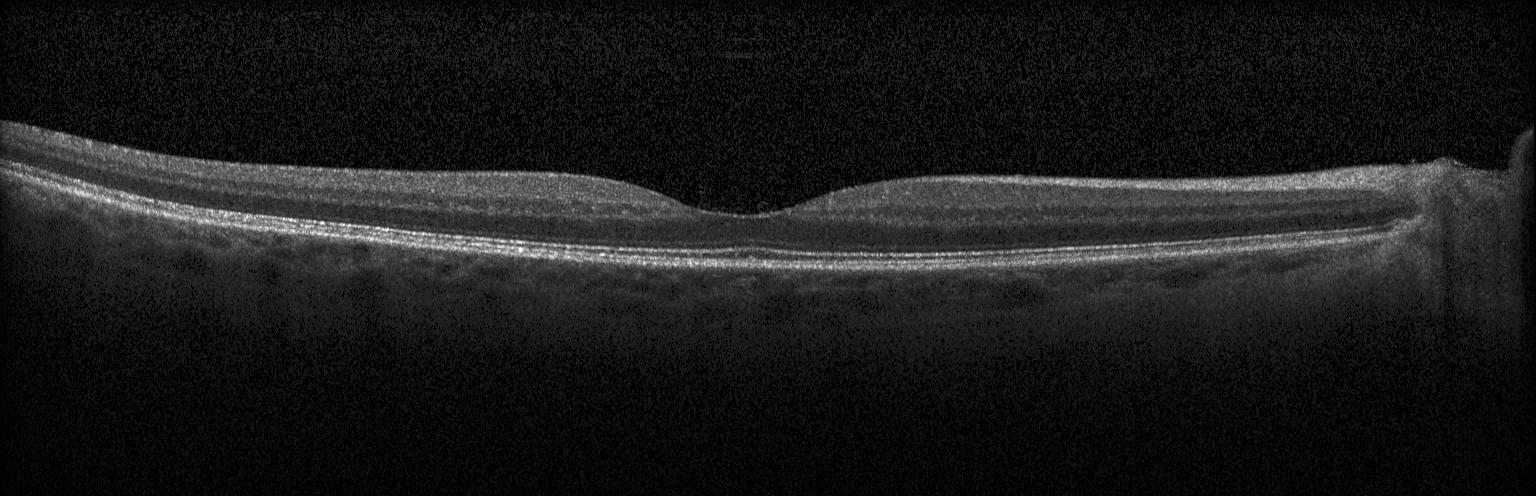

Impression: neither choroidal neovascularization, diabetic macular edema, nor drusen.